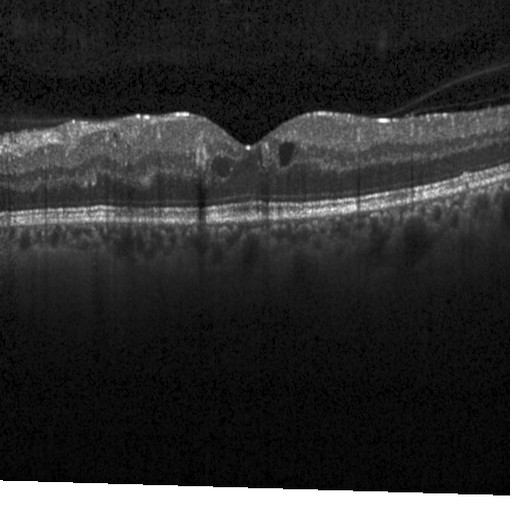 Acquired on a Heidelberg Spectralis · through the macula · OCT B-scan — Finding: diabetic macular edema.